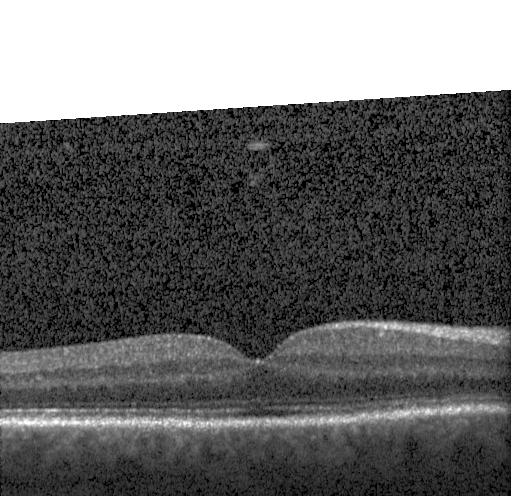
Spectral-domain optical coherence tomography; optical coherence tomography scan; Heidelberg Spectralis OCT system. Diagnosis: neither CNV, DME, nor drusen.